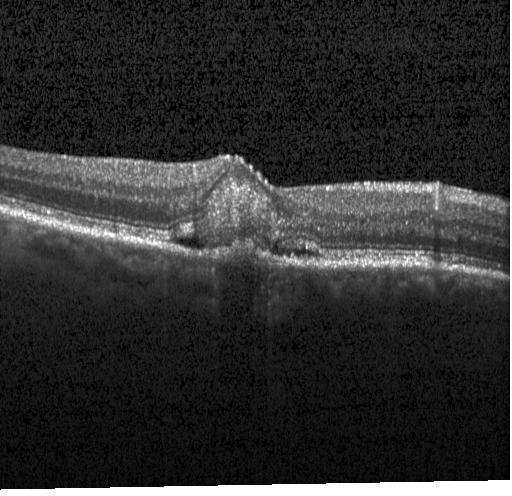

Finding: choroidal neovascularization (CNV).